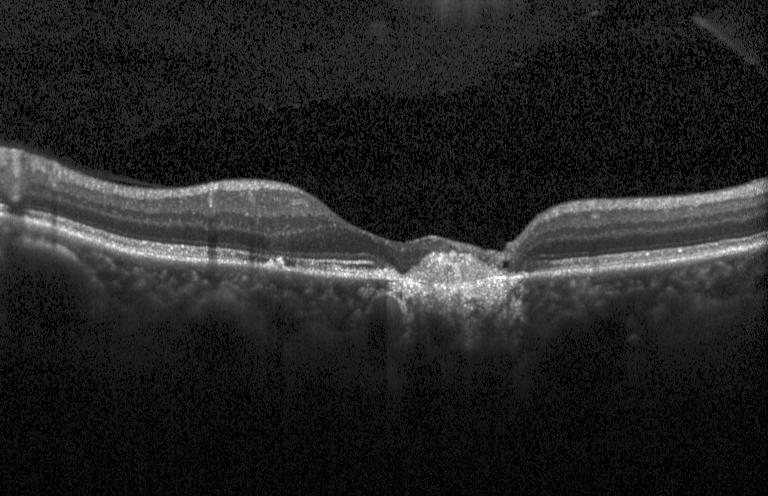

Heidelberg Spectralis OCT system, spectral-domain OCT, retinal OCT cross-section, centered on the fovea. The scan shows choroidal neovascularization.